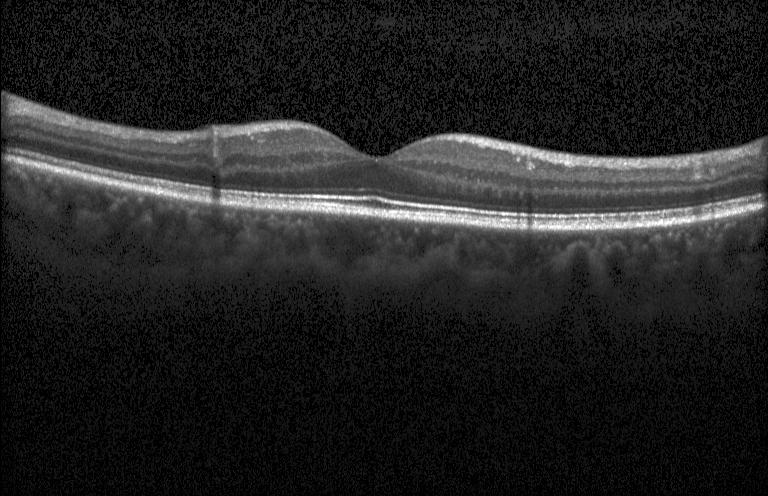

Retinal OCT B-scan, acquired on a Heidelberg Spectralis, SD-OCT, macular scan.
Finding: no CNV, DME, or drusen.